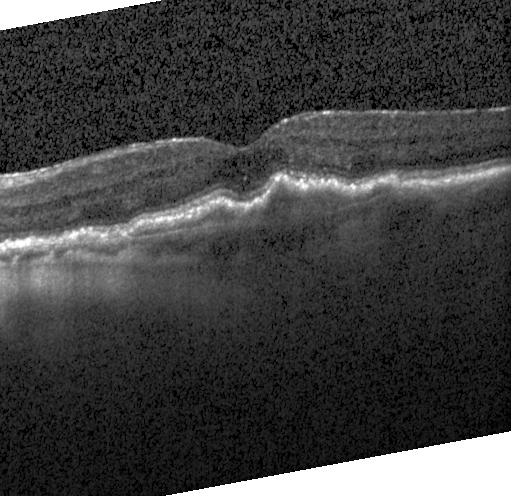

Heidelberg Spectralis; optical coherence tomography scan; horizontal scan through the fovea — Diagnosis: a choroidal neovascular membrane.